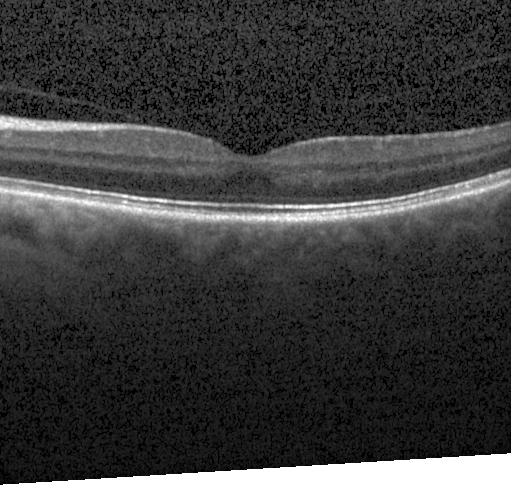 Heidelberg Spectralis OCT system · macular scan · retinal OCT B-scan · SD-OCT
The scan shows no choroidal neovascularization, no diabetic macular edema, and no drusen.